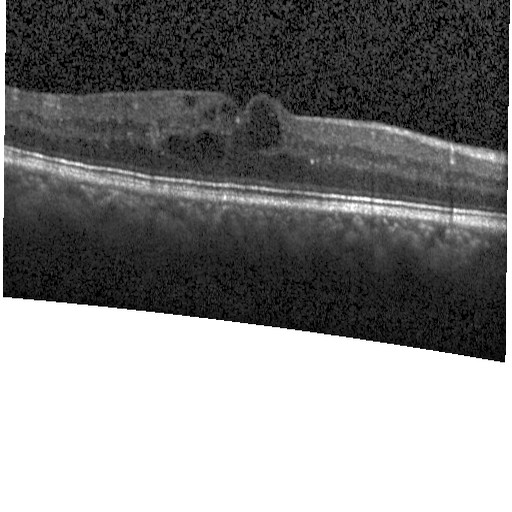
Retinal OCT B-scan; spectral-domain optical coherence tomography.
OCT finding: DME.